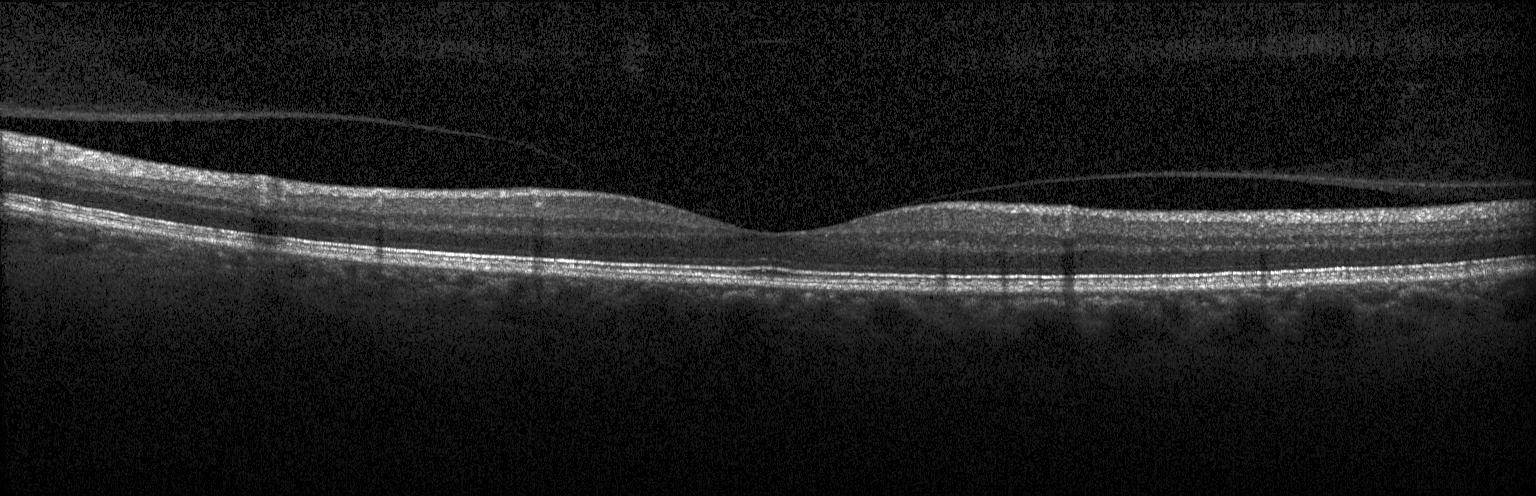 Retinal OCT cross-section — Assessment: no CNV, no DME, and no drusen.